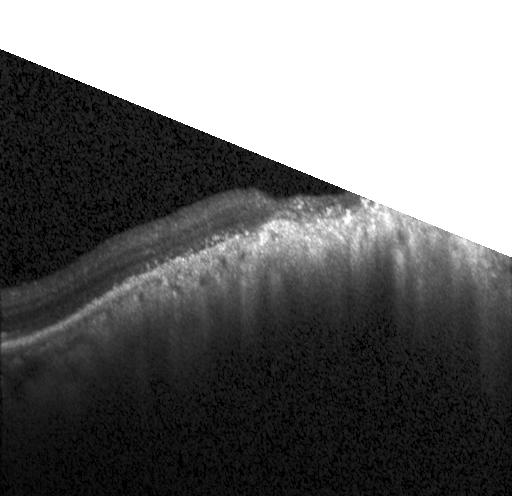 Optical coherence tomography B-scan — This B-scan demonstrates a choroidal neovascular membrane.